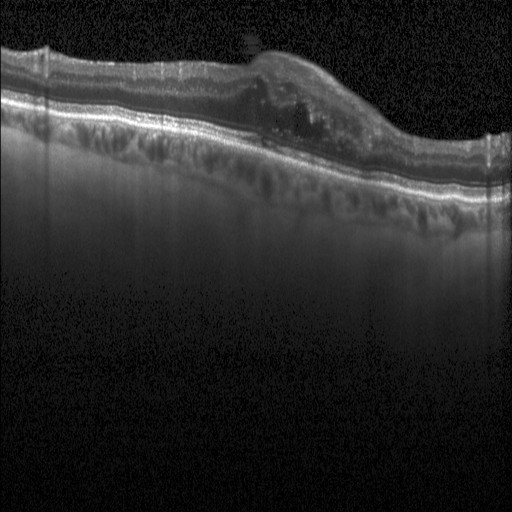 Retinal OCT cross-section, through the macula, spectral-domain OCT, Heidelberg Spectralis OCT system. Impression: diabetic macular edema.